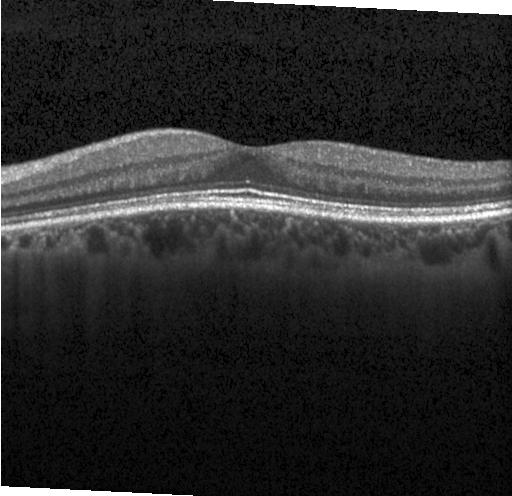
Macular scan, Heidelberg Spectralis OCT system, retinal OCT B-scan, spectral-domain OCT
Impression: no choroidal neovascularization, diabetic macular edema, or drusen.